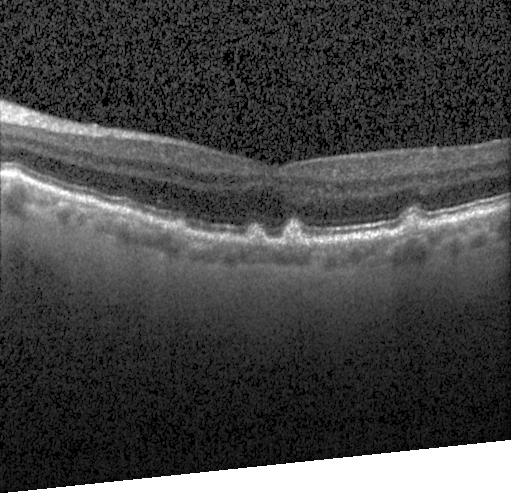
Optical coherence tomography B-scan.
Impression: drusen.